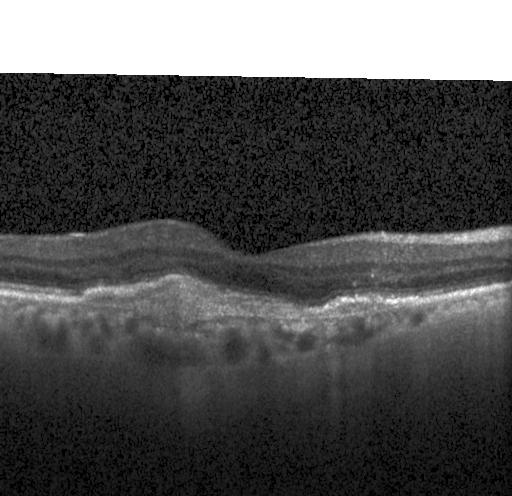 Acquired on a Heidelberg Spectralis · retinal OCT cross-section · spectral-domain optical coherence tomography · through the macula. A choroidal neovascular membrane.